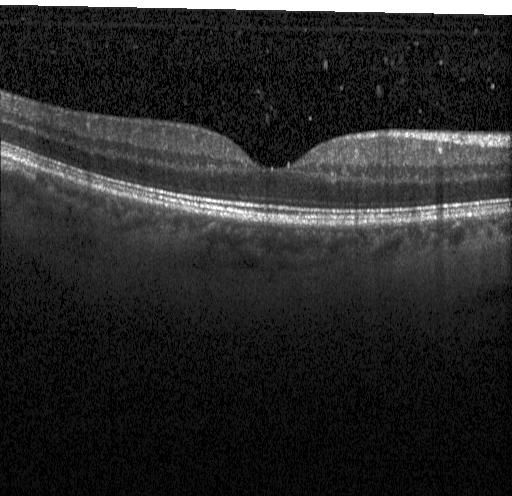 Optical coherence tomography scan.
Impression: no evidence of choroidal neovascularization, diabetic macular edema, or drusen.